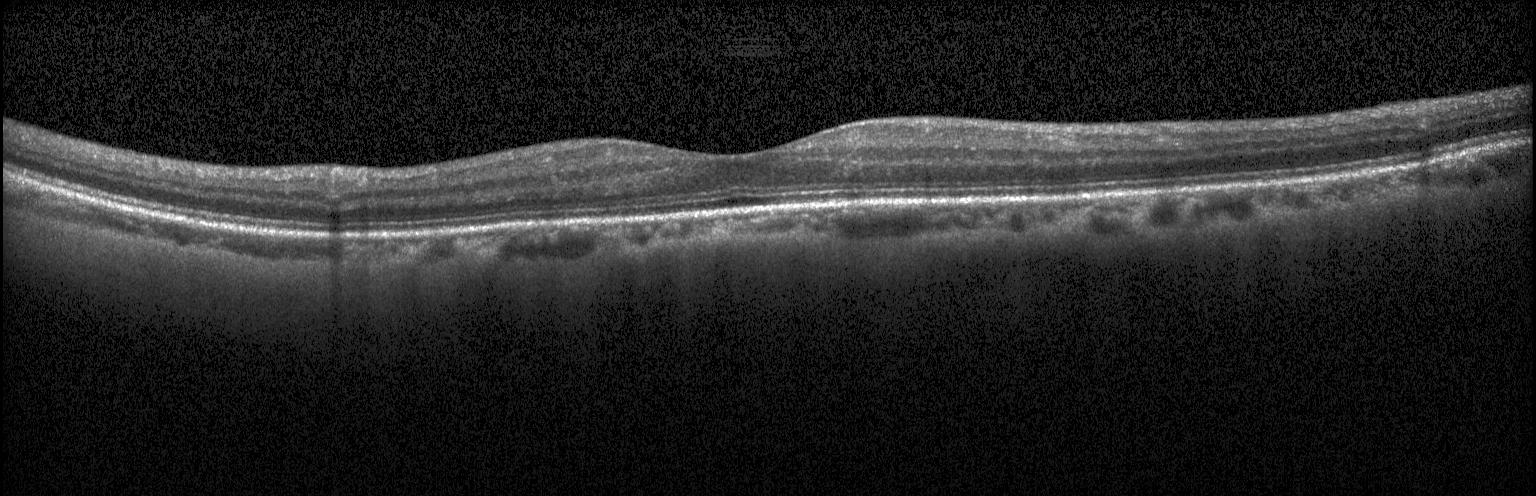
Optical coherence tomography B-scan, Heidelberg Spectralis OCT system.
Finding: no choroidal neovascularization, no diabetic macular edema, and no drusen.